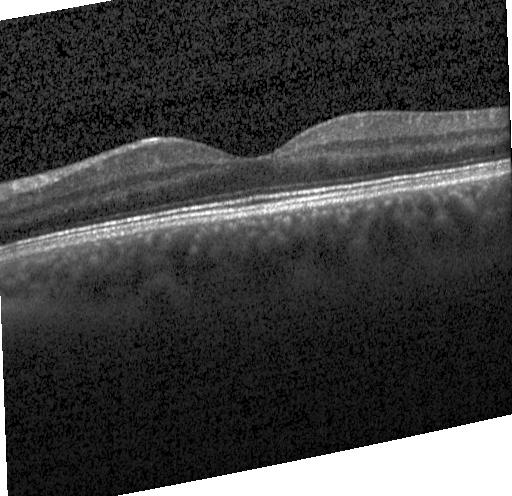

This B-scan demonstrates no choroidal neovascularization, diabetic macular edema, or drusen.